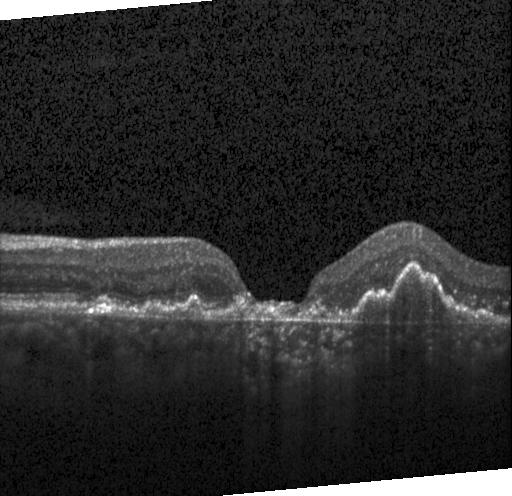

Retinal OCT cross-section. SD-OCT. Horizontal scan through the fovea
Assessment: choroidal neovascularization.